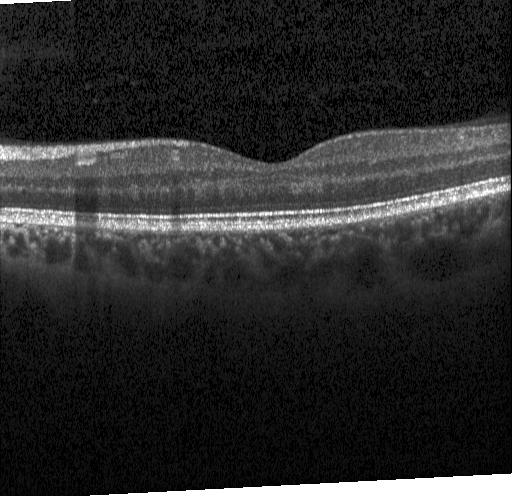 Retinal OCT B-scan. This B-scan demonstrates no CNV, DME, or drusen.